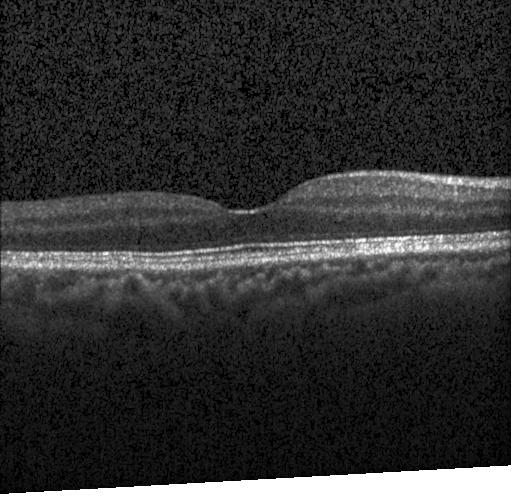
Fovea-centered, optical coherence tomography B-scan.
Diagnosis: neither choroidal neovascularization, diabetic macular edema, nor drusen.